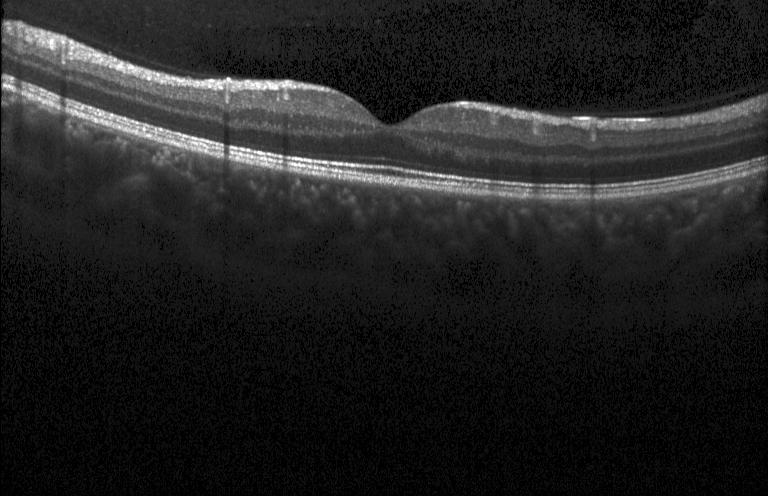
The scan shows no evidence of choroidal neovascularization, diabetic macular edema, or drusen.